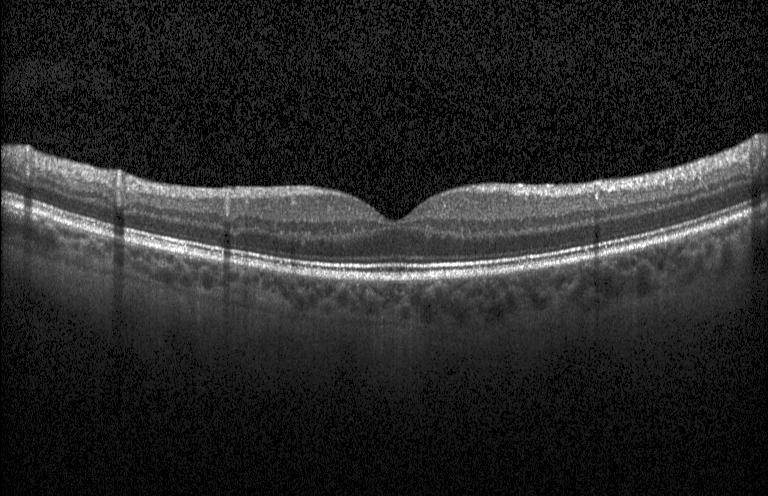 Through the macula. Acquired on a Heidelberg Spectralis. SD-OCT. Optical coherence tomography B-scan
OCT finding: neither choroidal neovascularization, diabetic macular edema, nor drusen.